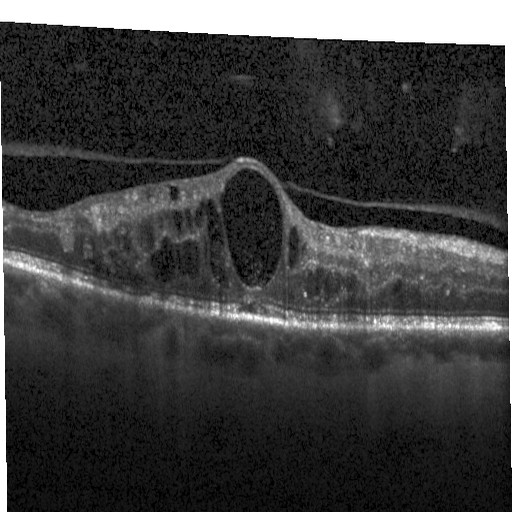

Fovea-centered. Instrument: Heidelberg Spectralis. Retinal OCT B-scan. Diagnosis: DME.